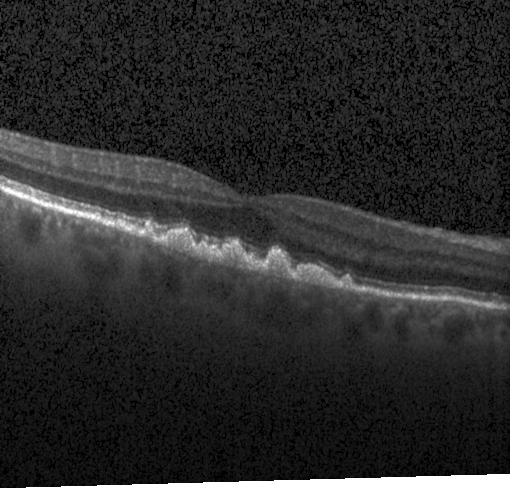 OCT line scan; macular scan — The scan shows multiple drusen.